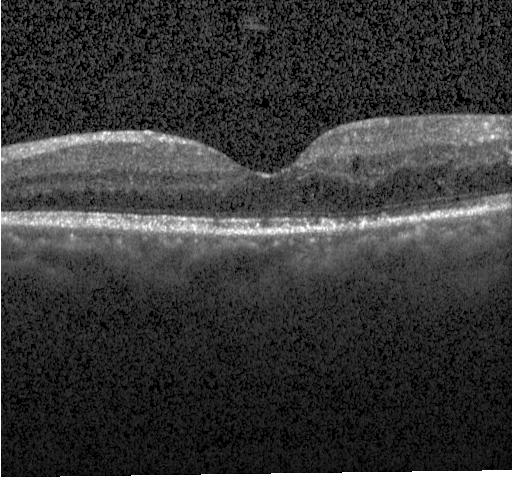
The scan shows diabetic macular edema.